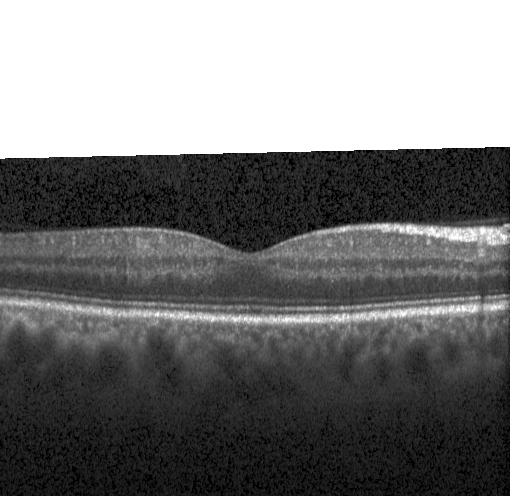
Retinal OCT cross-section. Impression: no CNV, no DME, and no drusen.